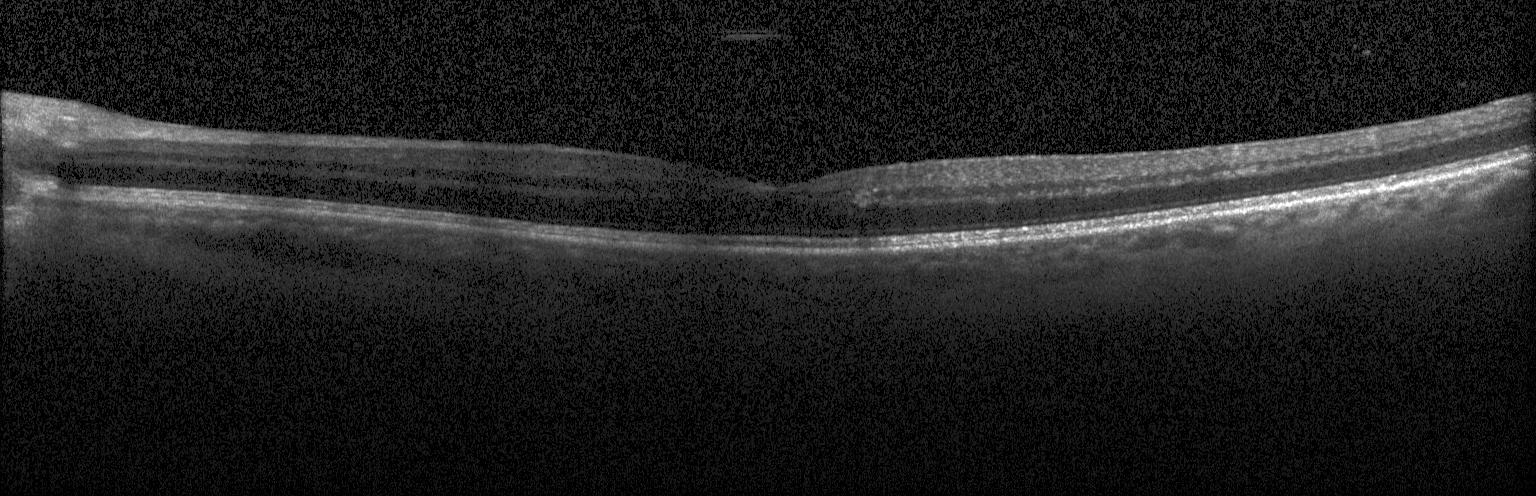
Dx: no CNV, DME, or drusen.